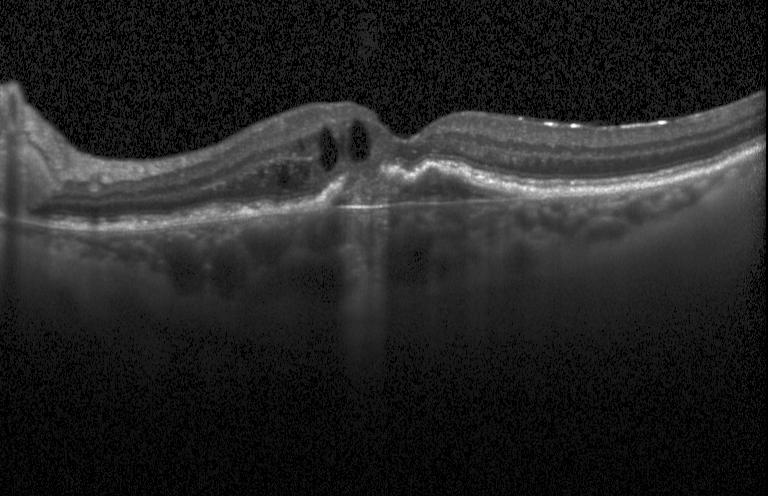 Impression: CNV.